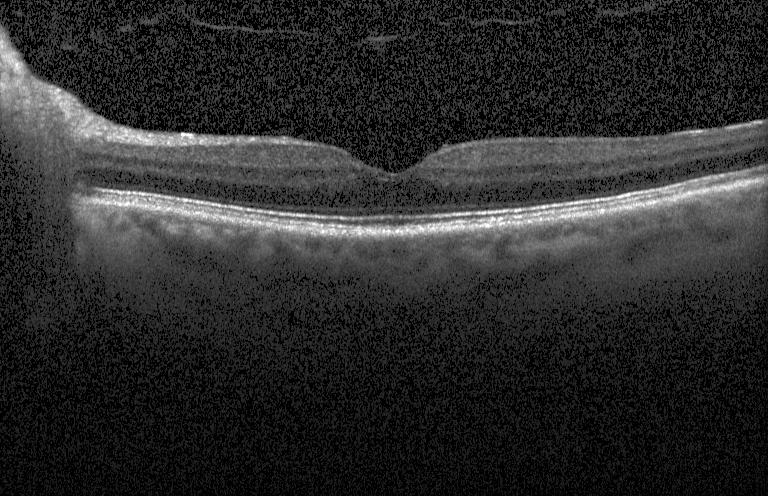
Macular OCT demonstrating neither CNV, DME, nor drusen.